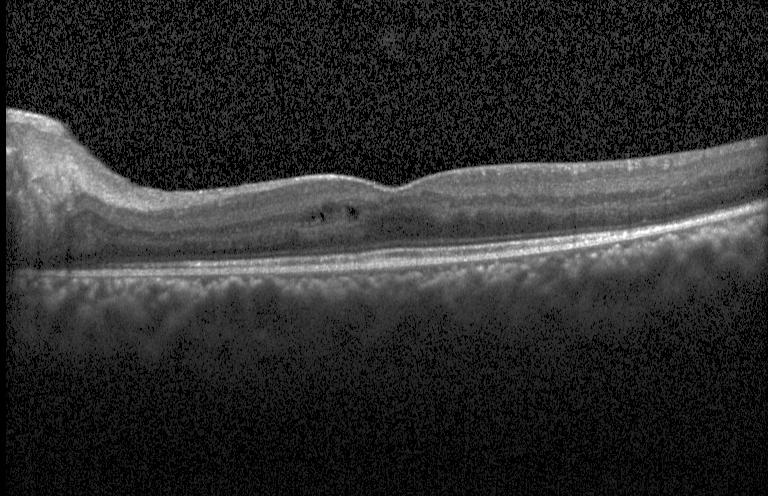

The scan shows diabetic macular edema (DME).